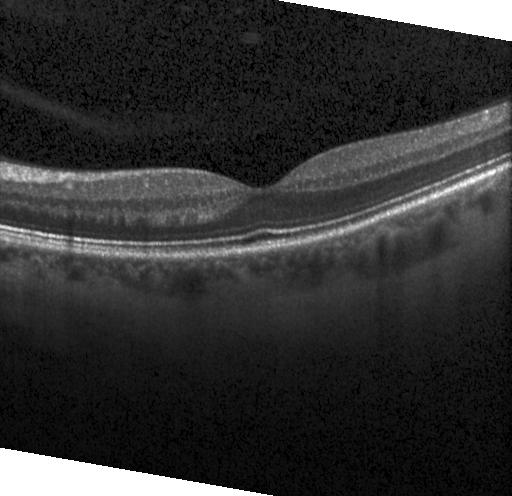

This B-scan demonstrates no CNV, DME, or drusen.